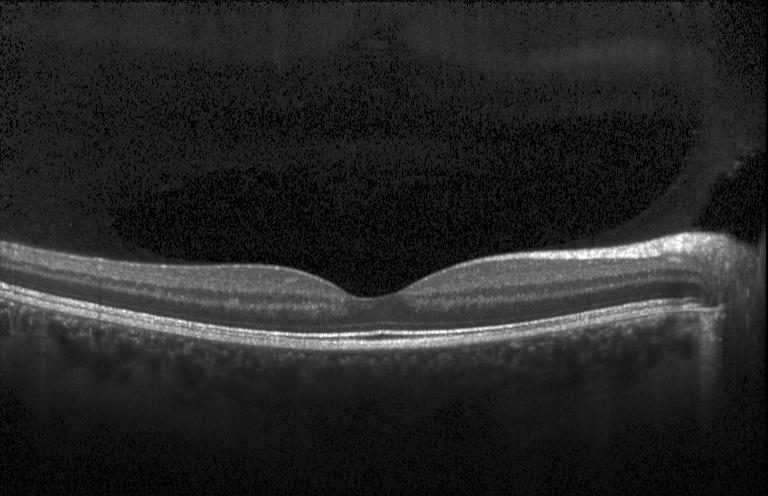 SD-OCT; fovea-centered; instrument: Heidelberg Spectralis; retinal OCT B-scan
Macular OCT: neither choroidal neovascularization, diabetic macular edema, nor drusen.